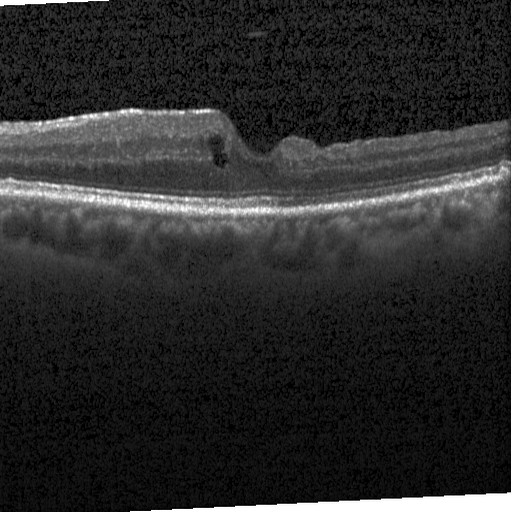

Diagnosis: DME.